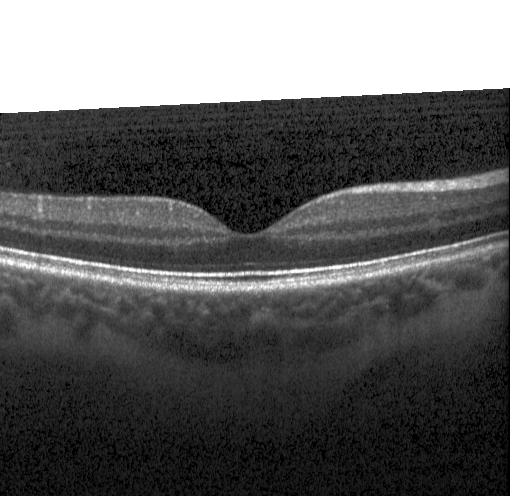

Through the macula; spectral-domain optical coherence tomography; retinal OCT cross-section
No evidence of CNV, DME, or drusen.